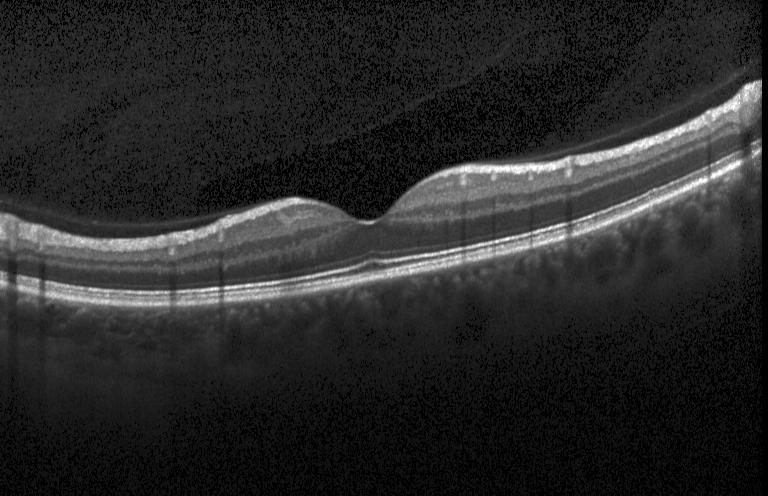
OCT B-scan · macular scan — Diagnosis: neither choroidal neovascularization, diabetic macular edema, nor drusen.